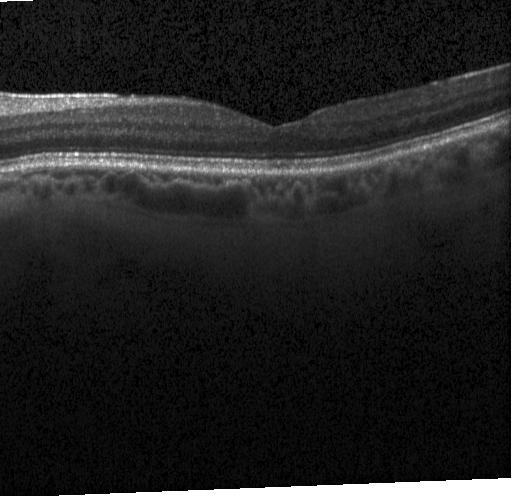

Finding: no CNV, no DME, and no drusen.